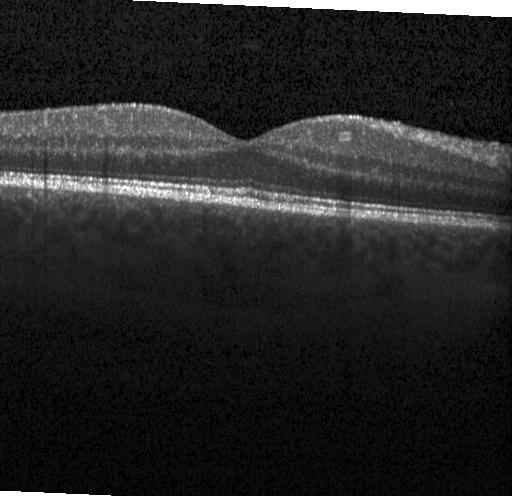

Retinal OCT cross-section. Heidelberg Spectralis. Centered on the fovea — Dx: no choroidal neovascularization, diabetic macular edema, or drusen.